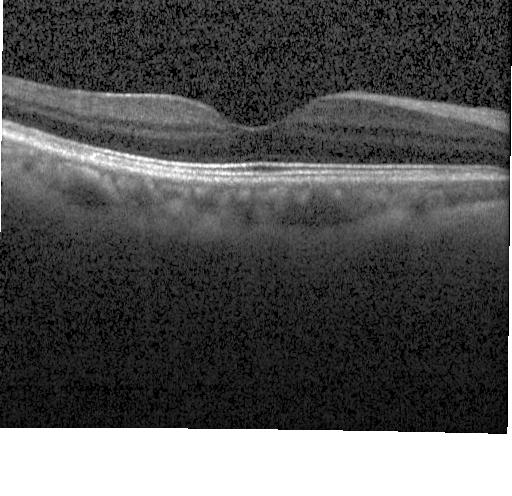 Through the macula · spectral-domain optical coherence tomography · optical coherence tomography scan · Heidelberg Spectralis OCT system — Diagnosis: no evidence of choroidal neovascularization, diabetic macular edema, or drusen.